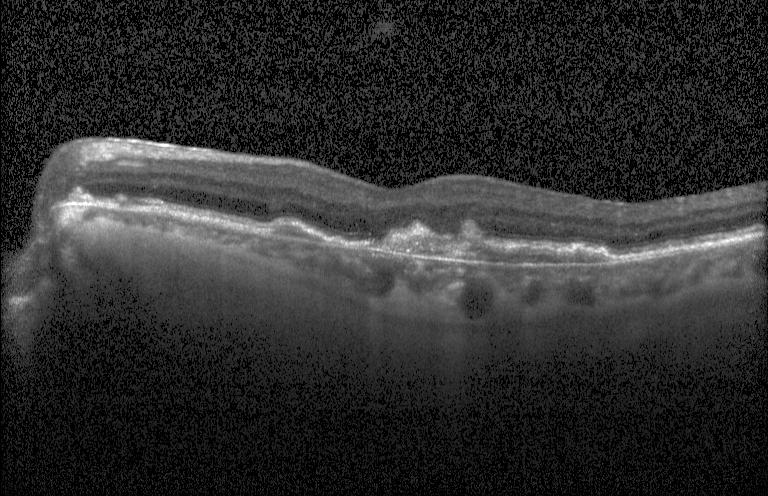
OCT finding: choroidal neovascularization (CNV).